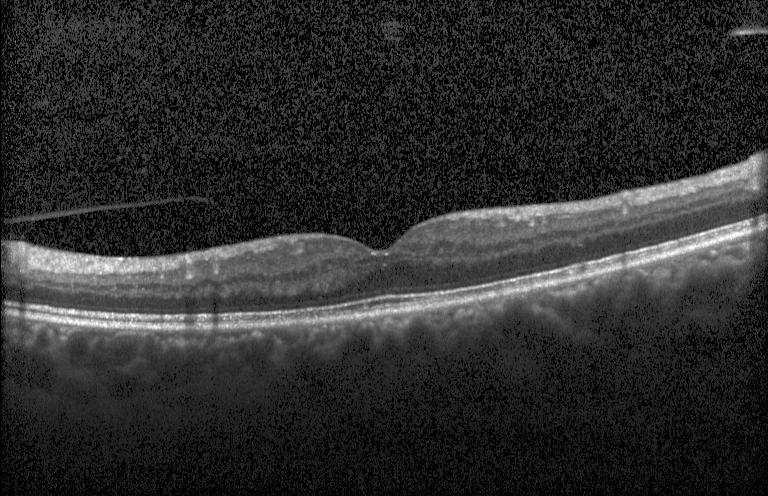
Assessment: neither choroidal neovascularization, diabetic macular edema, nor drusen.